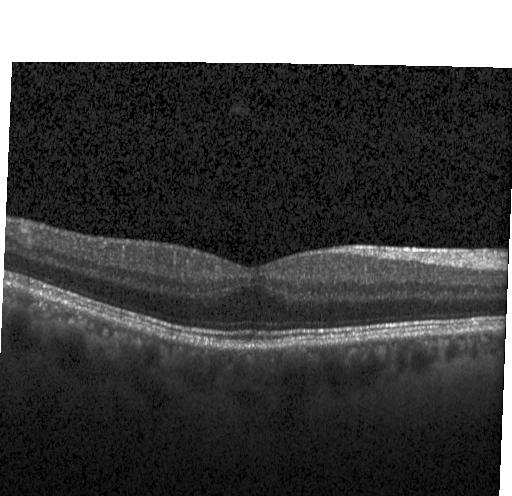

Horizontal scan through the fovea; Heidelberg Spectralis; optical coherence tomography B-scan. Impression: no choroidal neovascularization, diabetic macular edema, or drusen.